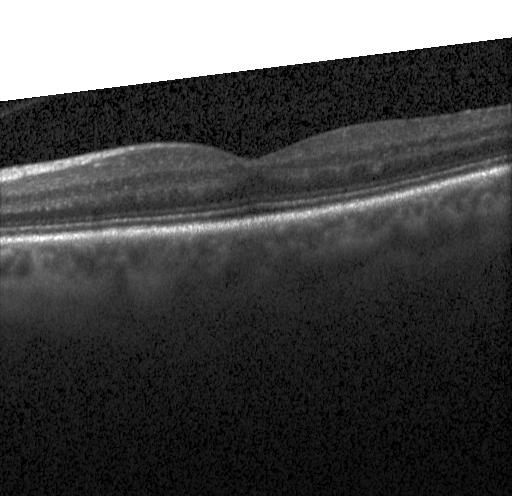 Macular OCT: neither choroidal neovascularization, diabetic macular edema, nor drusen.